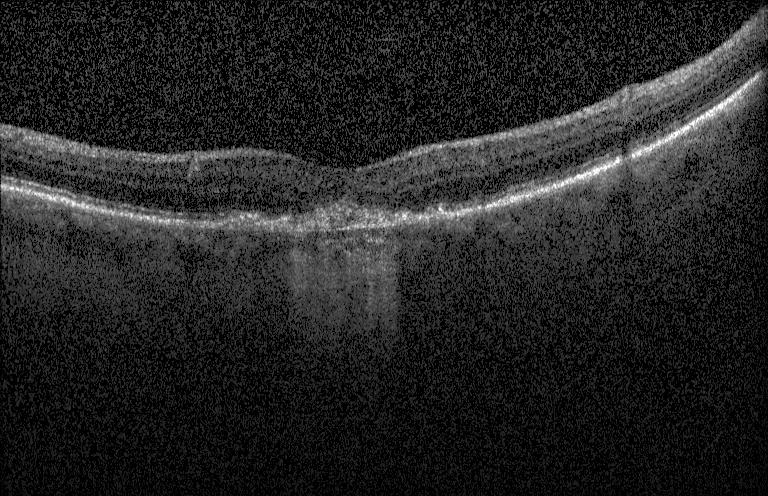

Retinal OCT B-scan. Diagnosis: a choroidal neovascular membrane.